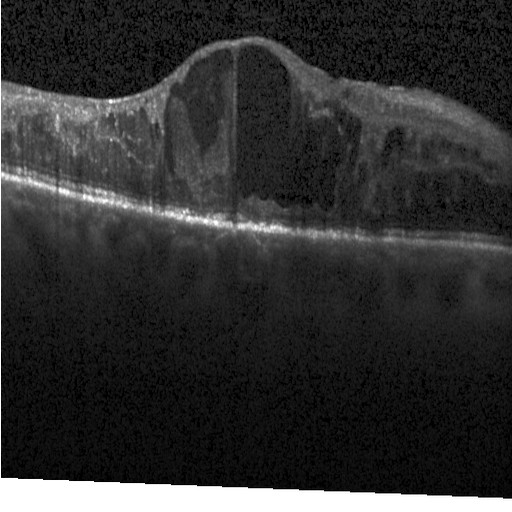
Optical coherence tomography B-scan. Through the macula.
Impression: diabetic macular edema.